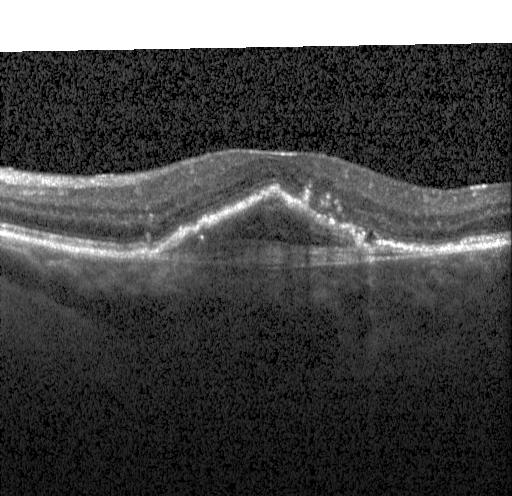
Optical coherence tomography scan. Through the macula. Spectral-domain OCT. Finding: choroidal neovascularization.